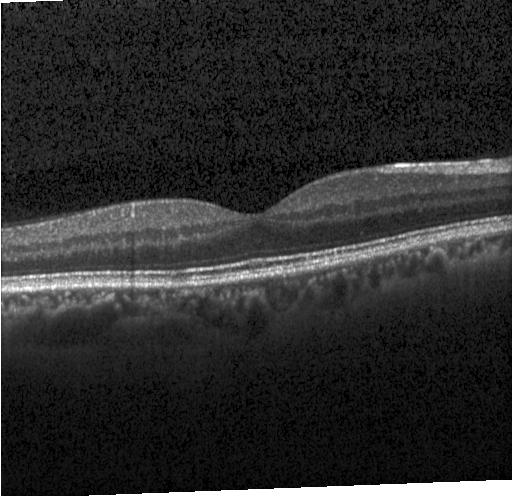
Optical coherence tomography scan. SD-OCT. Macular scan. Heidelberg Spectralis
Dx: no choroidal neovascularization, diabetic macular edema, or drusen.